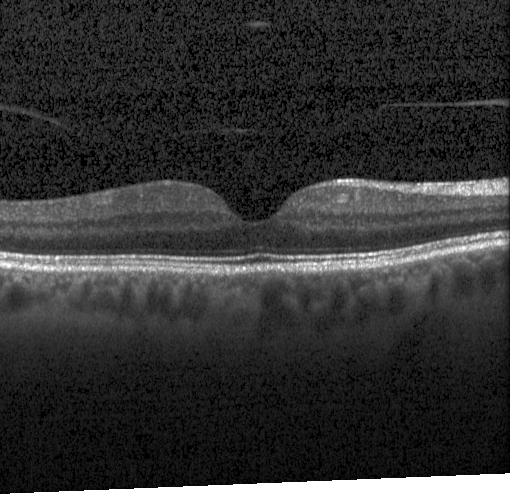

Optical coherence tomography scan — Macular OCT: no CNV, no DME, and no drusen.